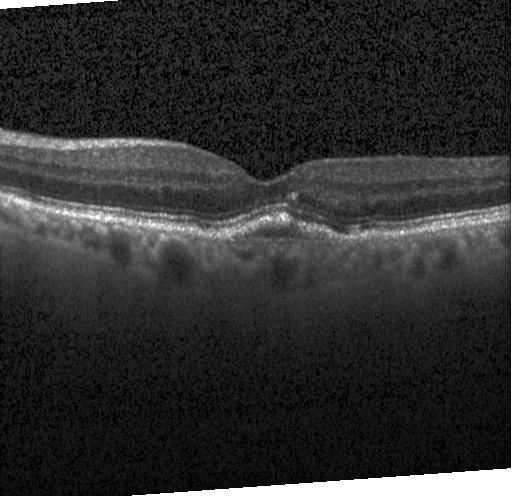
Optical coherence tomography B-scan.
Impression: a choroidal neovascular membrane.